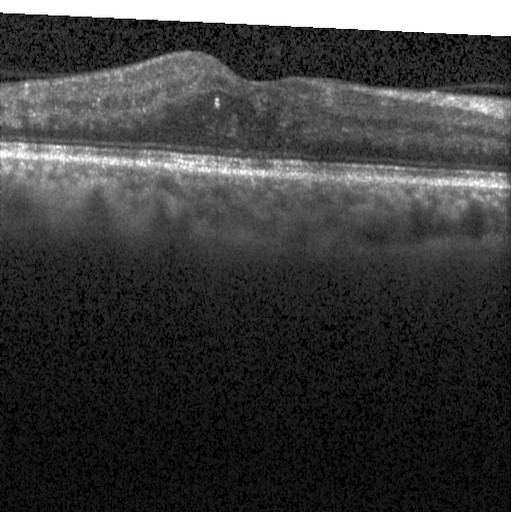 Fovea-centered; SD-OCT; OCT B-scan. Impression: DME.